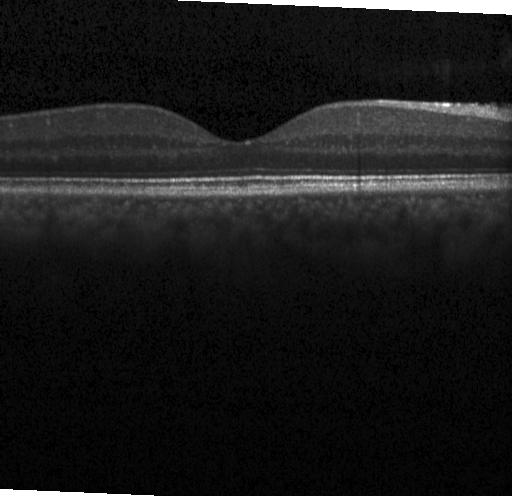

Finding: no choroidal neovascularization, diabetic macular edema, or drusen.